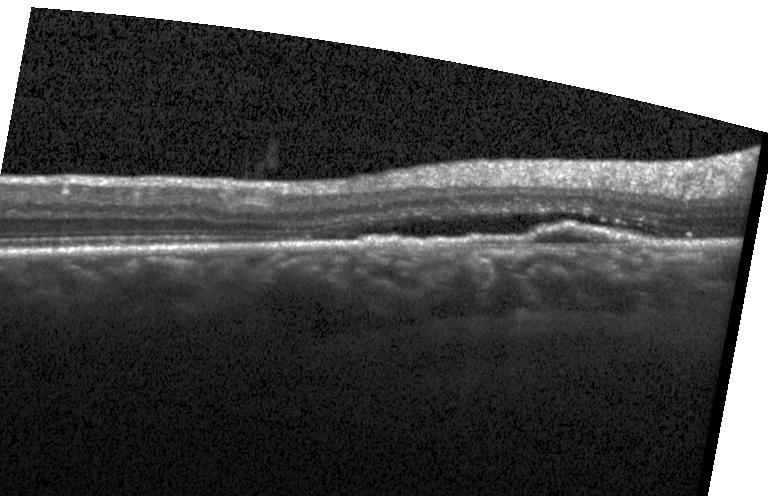

Optical coherence tomography B-scan. OCT finding: a choroidal neovascular membrane.